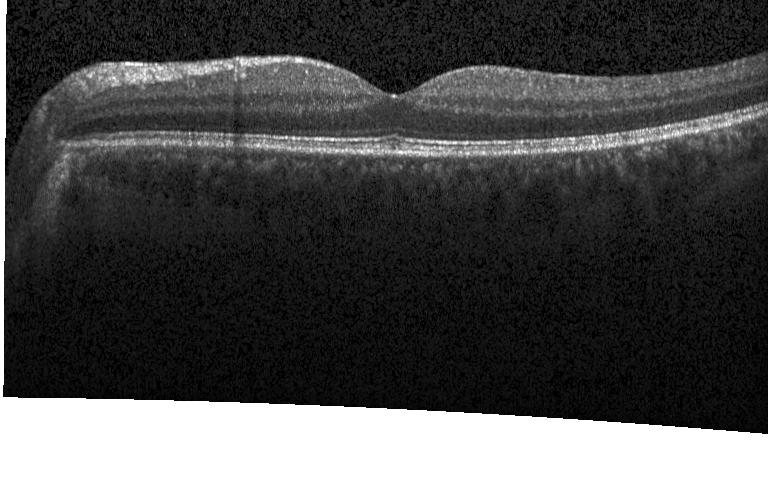

Spectral-domain optical coherence tomography, retinal OCT B-scan.
Impression: neither choroidal neovascularization, diabetic macular edema, nor drusen.